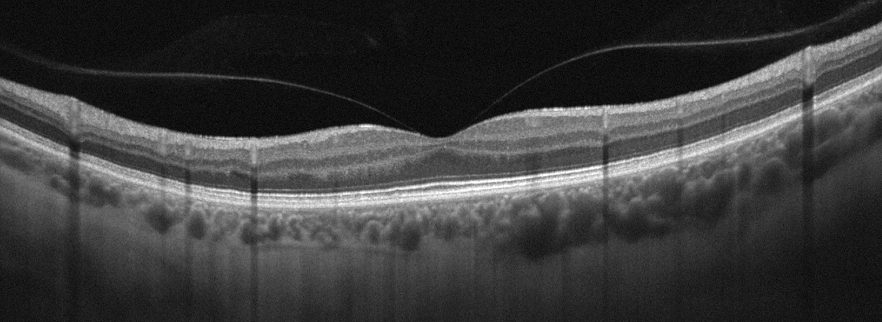 Right eye · optical coherence tomography B-scan.
Assessment: epiretinal membrane.